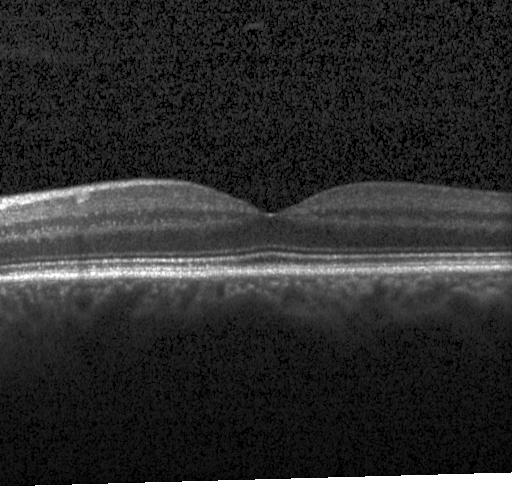
Optical coherence tomography scan — Finding: no choroidal neovascularization, diabetic macular edema, or drusen.